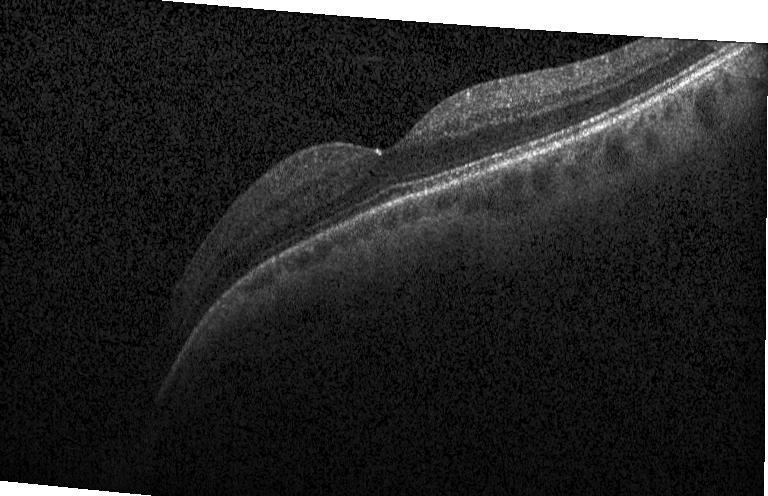
Through the macula. OCT line scan. Spectral-domain OCT. Heidelberg Spectralis OCT system — The scan shows no CNV, no DME, and no drusen.